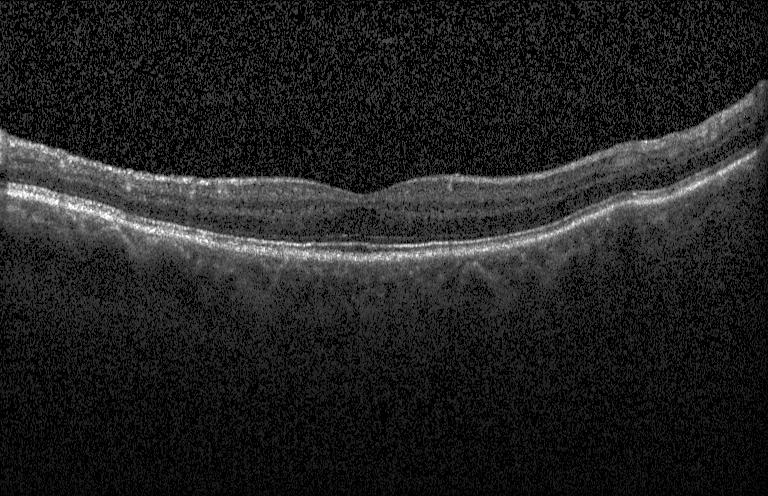
Impression: neither choroidal neovascularization, diabetic macular edema, nor drusen.